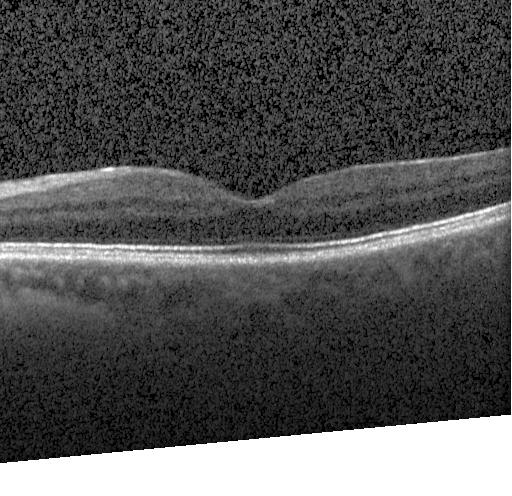
OCT B-scan showing no evidence of CNV, DME, or drusen.